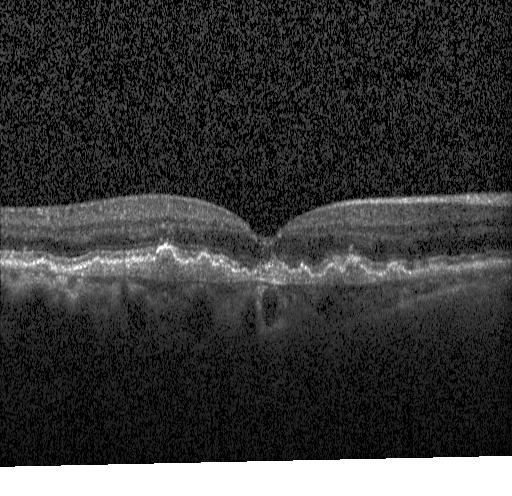 Retinal OCT B-scan, acquired on a Heidelberg Spectralis, macular scan, spectral-domain optical coherence tomography.
Diagnosis: choroidal neovascularization.